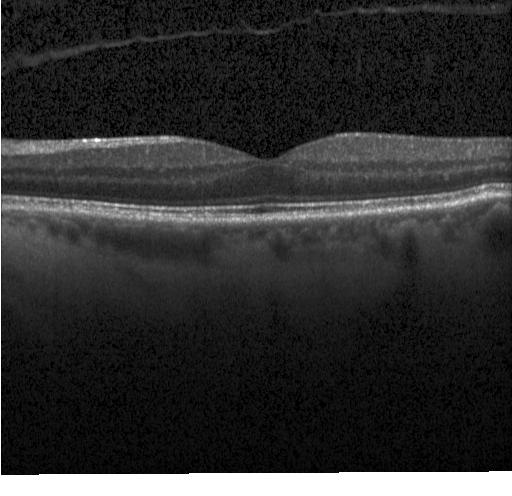 Horizontal scan through the fovea · instrument: Heidelberg Spectralis · spectral-domain OCT · retinal OCT B-scan. Impression: no choroidal neovascularization, no diabetic macular edema, and no drusen.